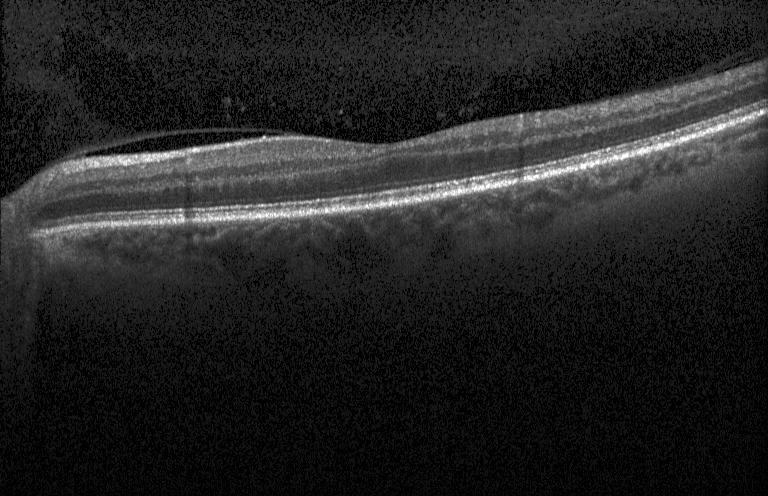
Retinal OCT cross-section, Heidelberg Spectralis OCT system
Assessment: neither CNV, DME, nor drusen.